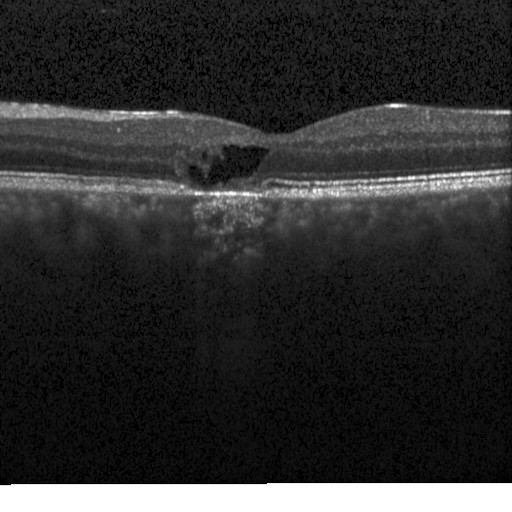

Horizontal scan through the fovea; acquired on a Heidelberg Spectralis; optical coherence tomography B-scan. Finding: DME.